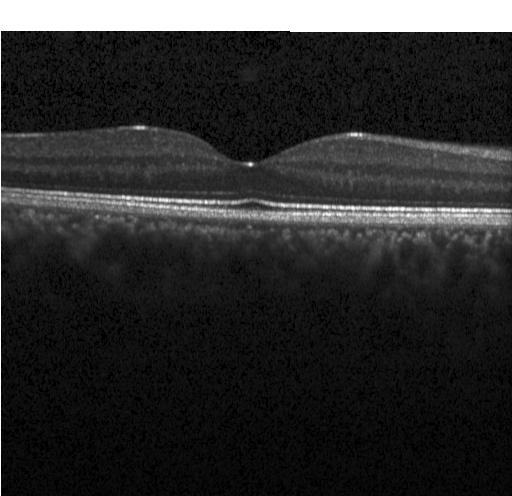

OCT finding: no choroidal neovascularization, diabetic macular edema, or drusen.